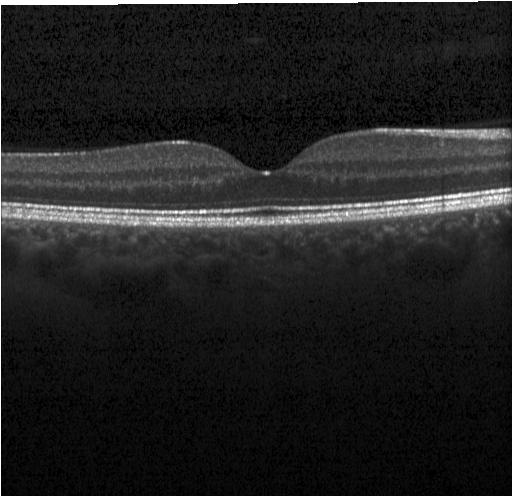
Optical coherence tomography B-scan. SD-OCT. Fovea-centered.
Diagnosis: no evidence of choroidal neovascularization, diabetic macular edema, or drusen.